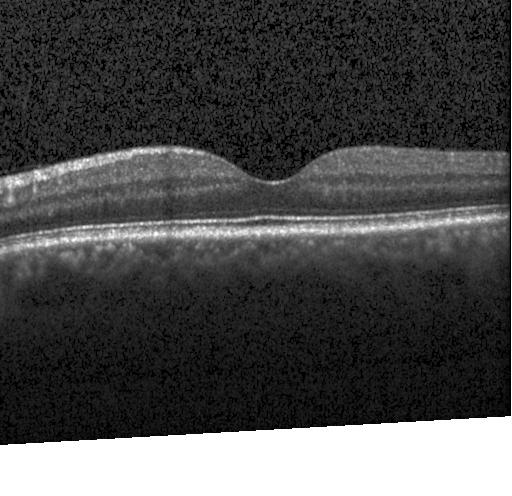
Macular OCT: neither choroidal neovascularization, diabetic macular edema, nor drusen.